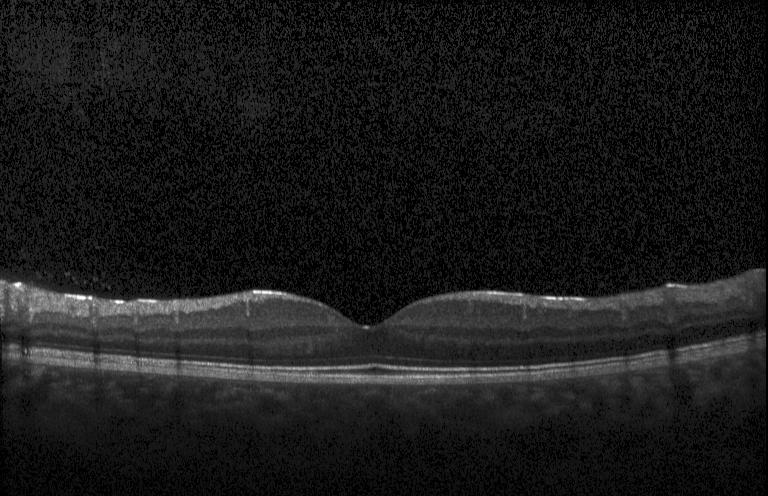

Acquired on a Heidelberg Spectralis · fovea-centered · OCT B-scan · spectral-domain optical coherence tomography. This B-scan demonstrates no choroidal neovascularization, no diabetic macular edema, and no drusen.